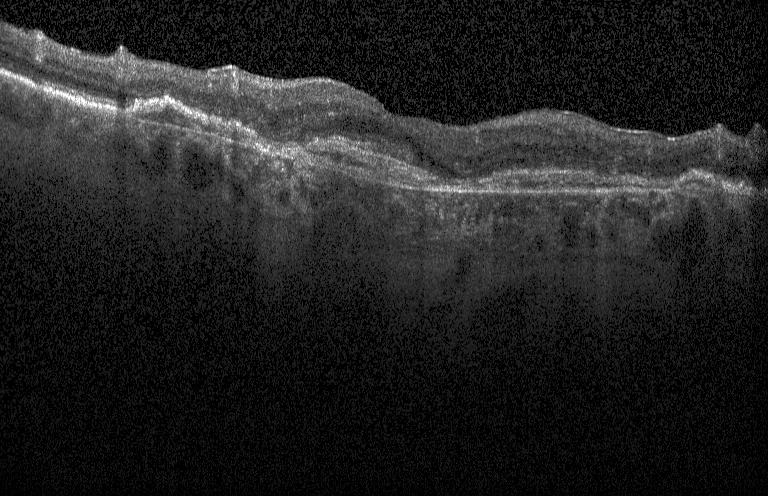

Optical coherence tomography B-scan
Finding: a choroidal neovascular membrane.